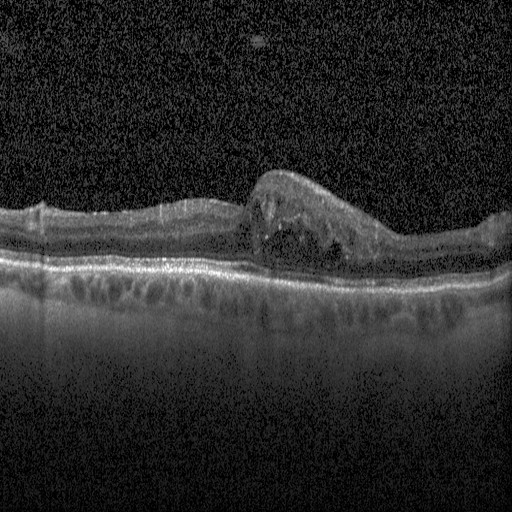
Through the macula. Spectral-domain optical coherence tomography. Heidelberg Spectralis OCT system. Retinal OCT cross-section — This B-scan demonstrates diabetic macular edema (DME).